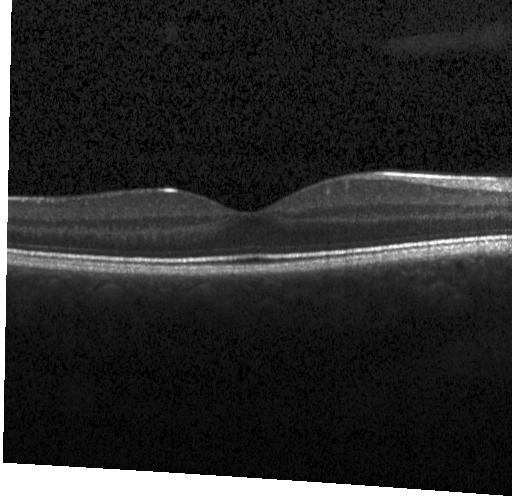

Optical coherence tomography scan, instrument: Heidelberg Spectralis, spectral-domain optical coherence tomography — OCT finding: no choroidal neovascularization, diabetic macular edema, or drusen.